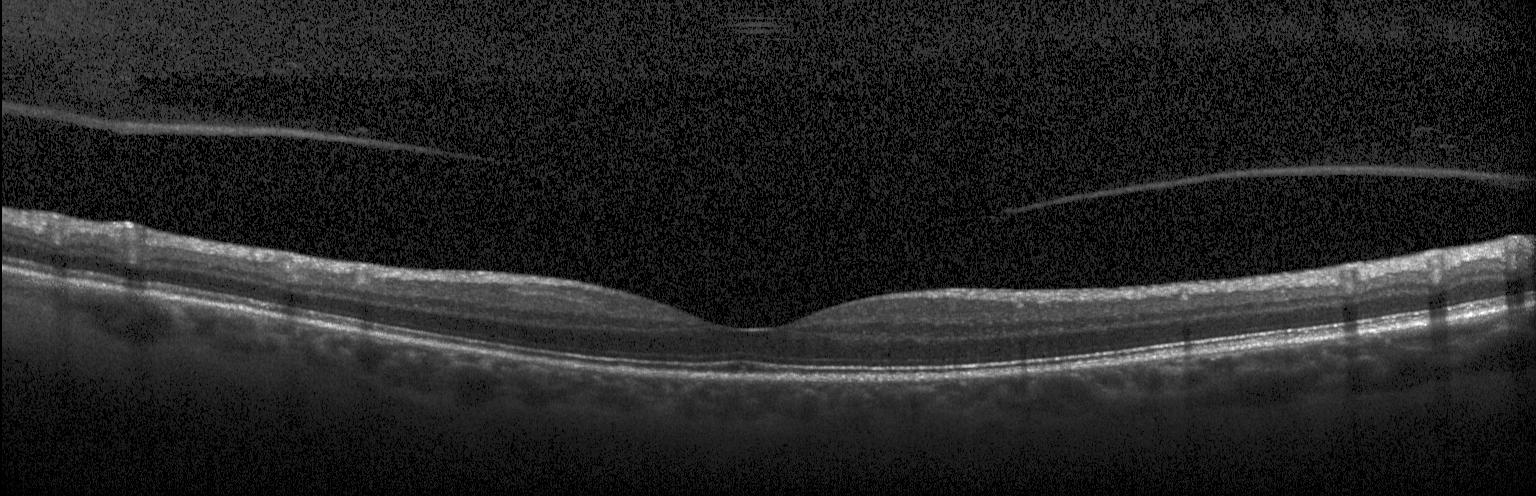
OCT B-scan showing no choroidal neovascularization, diabetic macular edema, or drusen.